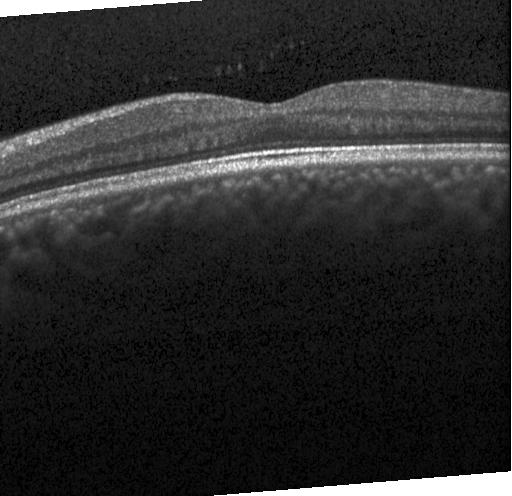

Retinal OCT B-scan, SD-OCT, through the macula, acquired on a Heidelberg Spectralis. Impression: no choroidal neovascularization, no diabetic macular edema, and no drusen.